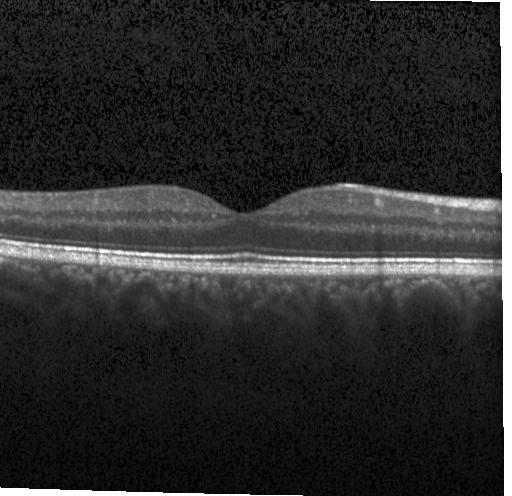

OCT line scan · acquired on a Heidelberg Spectralis · spectral-domain OCT · fovea-centered
The scan shows no choroidal neovascularization, no diabetic macular edema, and no drusen.